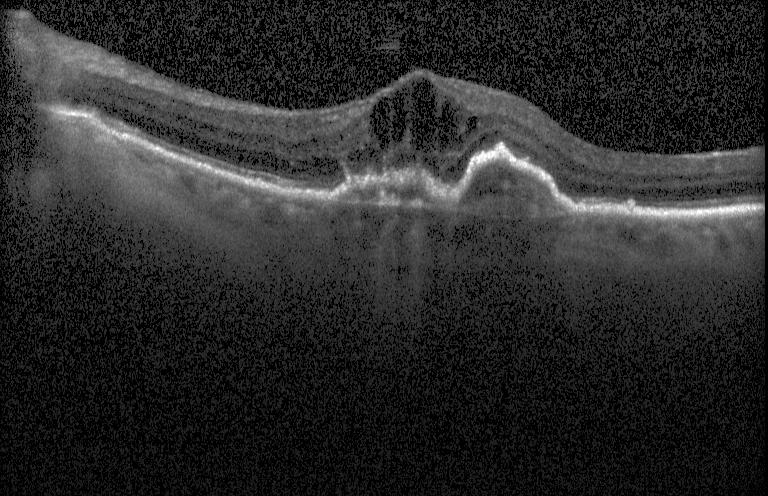

This B-scan demonstrates choroidal neovascularization (CNV).